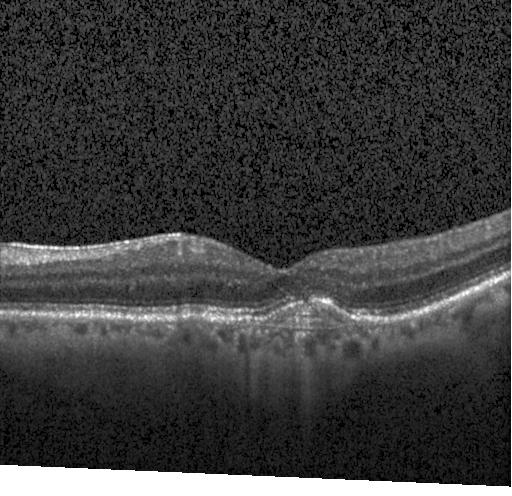

SD-OCT, acquired on a Heidelberg Spectralis, retinal OCT cross-section, fovea-centered.
The scan shows CNV.